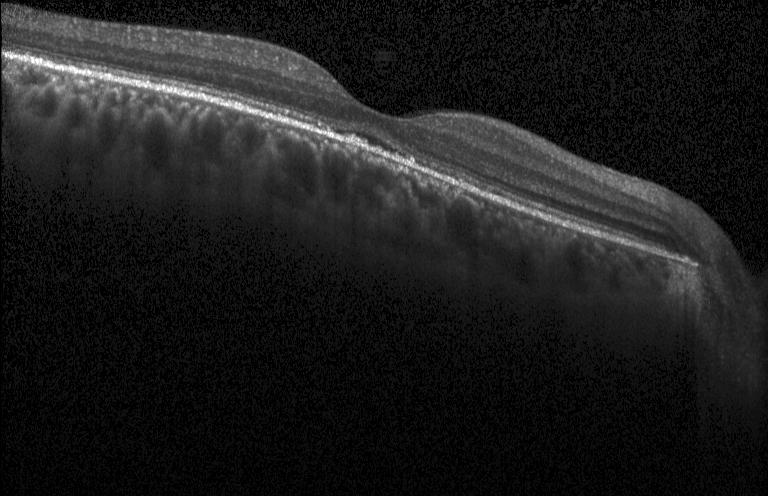 Diagnosis: no CNV, DME, or drusen.